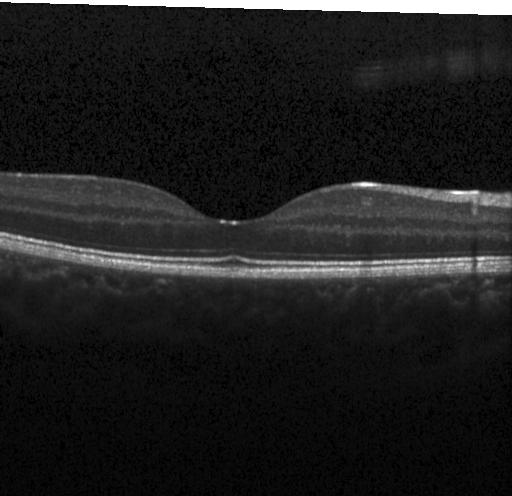 Acquired on a Heidelberg Spectralis. Spectral-domain OCT. Fovea-centered. Optical coherence tomography B-scan. Diagnosis: neither choroidal neovascularization, diabetic macular edema, nor drusen.